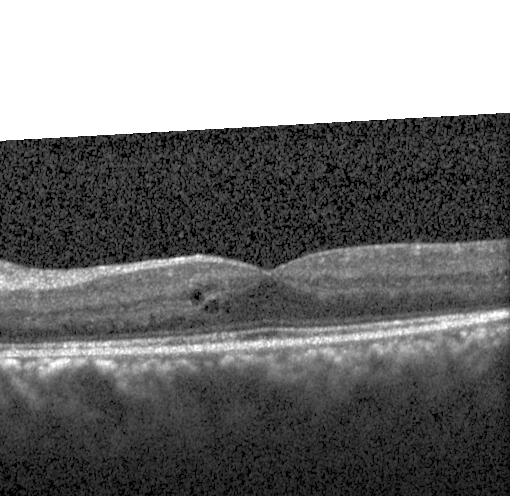 DME.